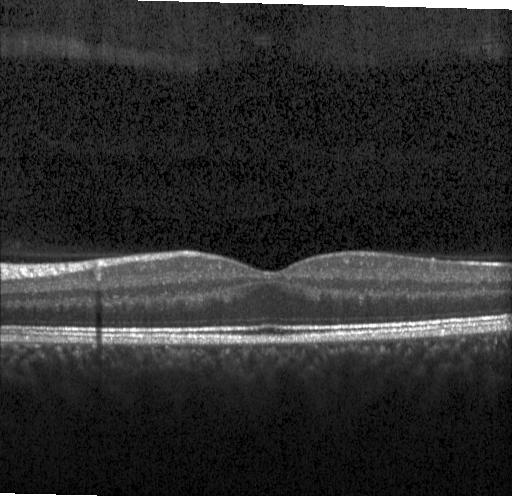 Through the macula · Heidelberg Spectralis OCT system · SD-OCT · retinal OCT B-scan
Finding: neither choroidal neovascularization, diabetic macular edema, nor drusen.